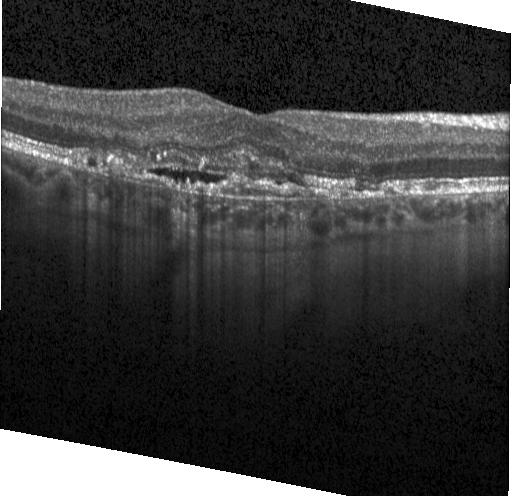
Optical coherence tomography scan
Impression: a choroidal neovascular membrane.